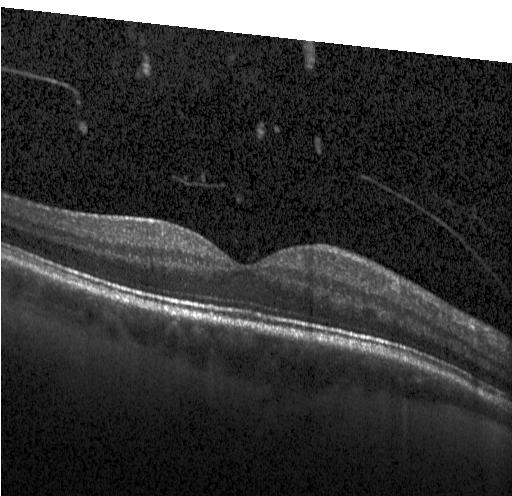

Macular OCT: no choroidal neovascularization, diabetic macular edema, or drusen.